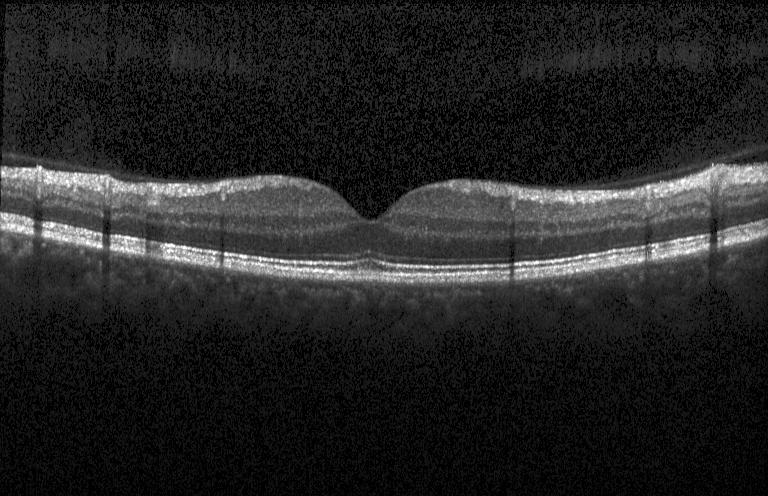

OCT finding: neither choroidal neovascularization, diabetic macular edema, nor drusen.